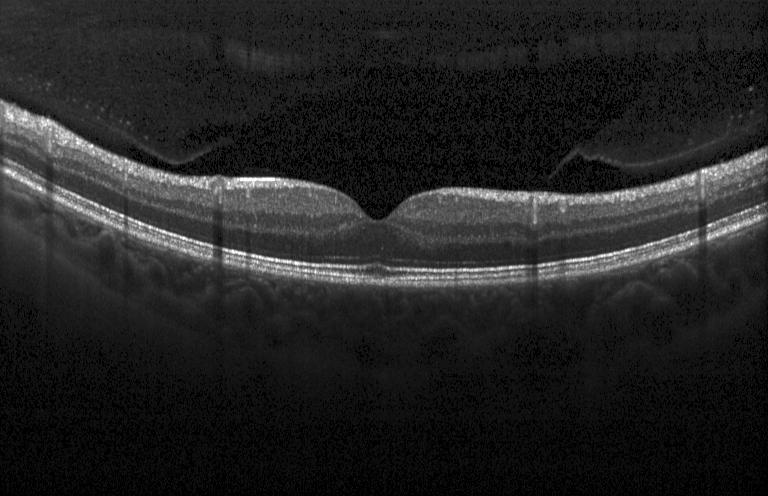

OCT scan showing no choroidal neovascularization, diabetic macular edema, or drusen.